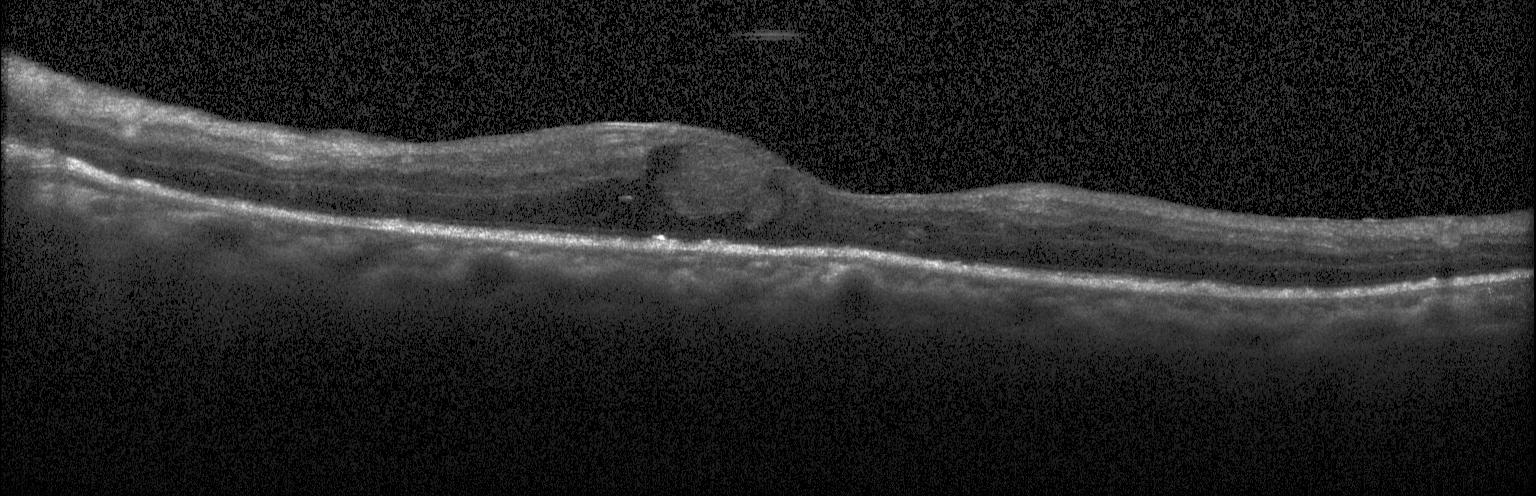 OCT finding: DME.